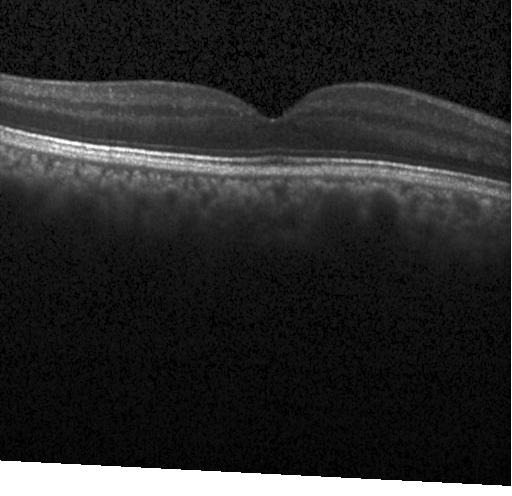 Retinal OCT B-scan.
The scan shows no CNV, DME, or drusen.